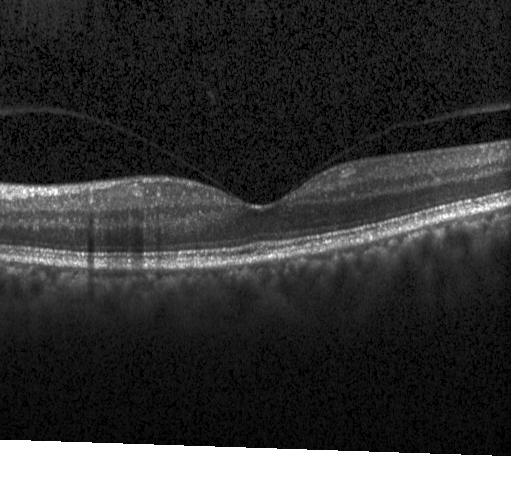

Spectral-domain OCT B-scan: no CNV, DME, or drusen.